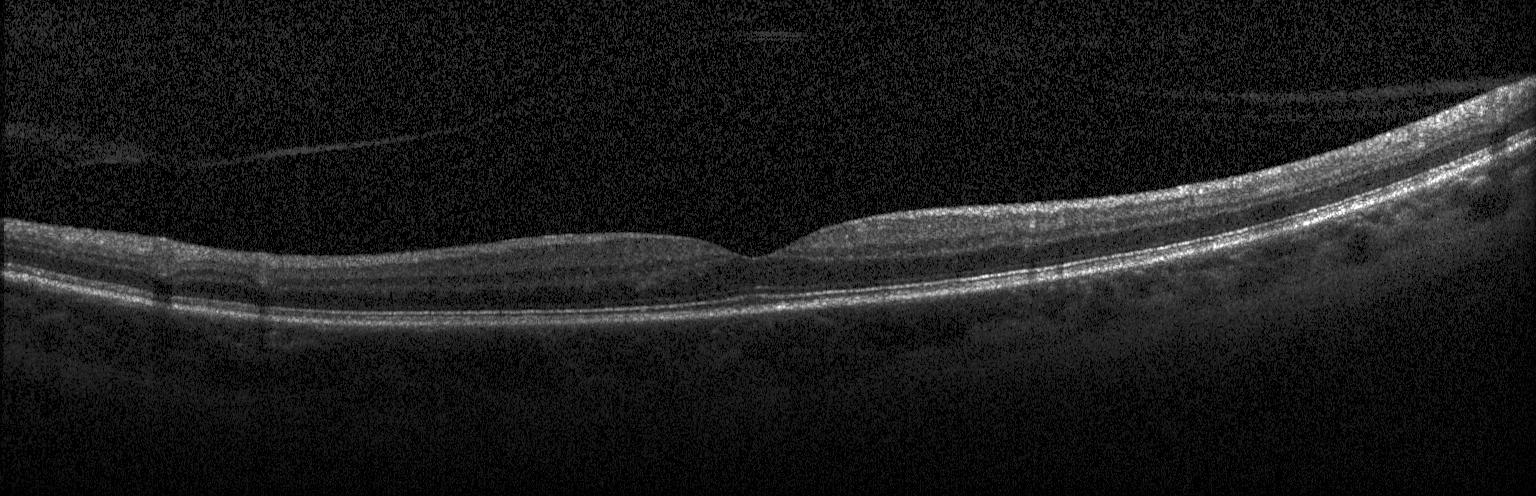

Retinal OCT cross-section. Heidelberg Spectralis OCT system. Through the macula — No CNV, DME, or drusen.